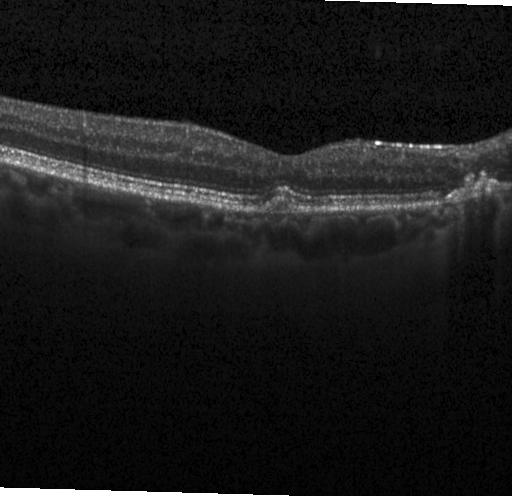
Heidelberg Spectralis; OCT line scan; SD-OCT — Diagnosis: choroidal neovascularization.